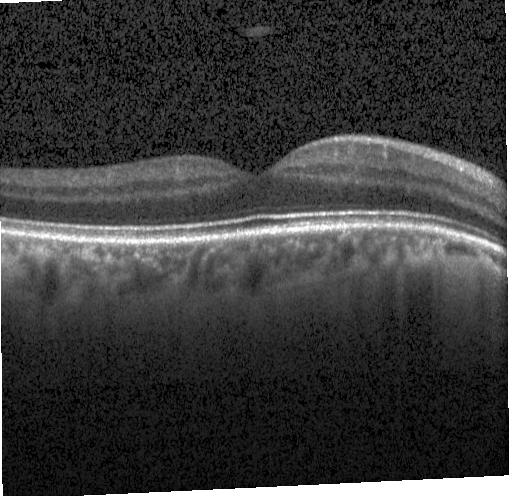 Spectral-domain optical coherence tomography, optical coherence tomography B-scan, Heidelberg Spectralis OCT system — No choroidal neovascularization, diabetic macular edema, or drusen.